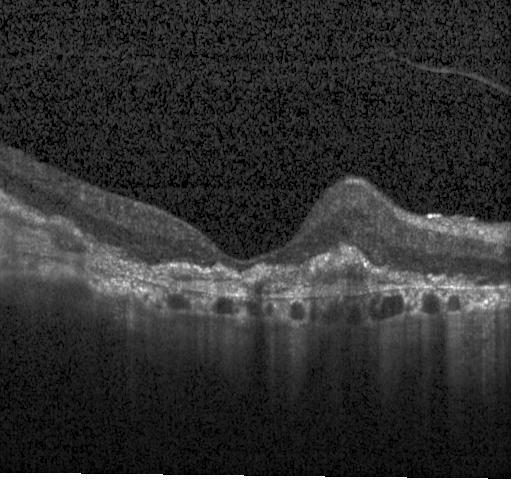

Retinal OCT B-scan; SD-OCT; acquired on a Heidelberg Spectralis; macular scan.
Diagnosis: choroidal neovascularization (CNV).